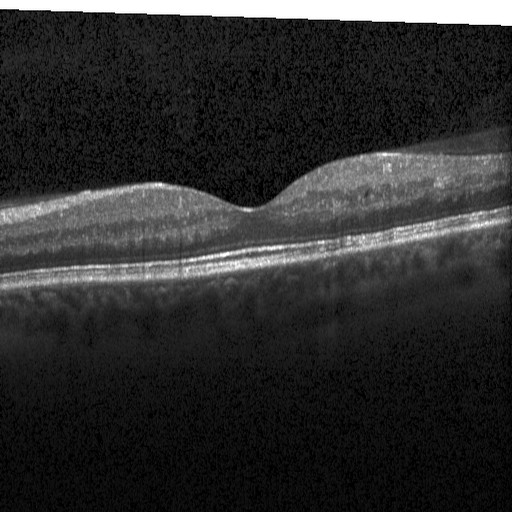 Acquired on a Heidelberg Spectralis · spectral-domain OCT · optical coherence tomography B-scan · horizontal scan through the fovea. Finding: diabetic macular edema.